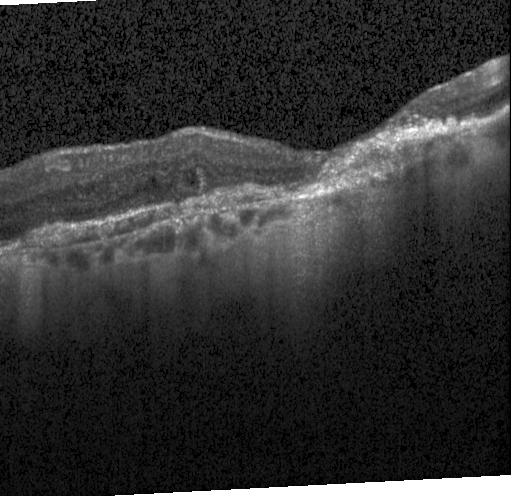 Impression: choroidal neovascularization.